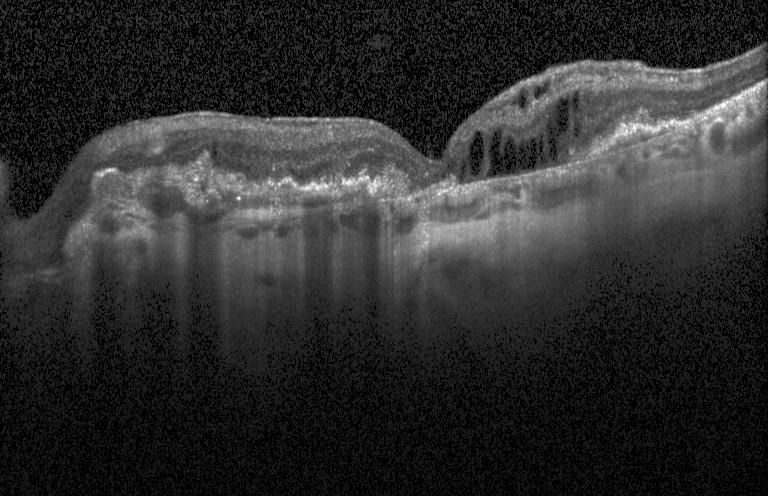

Retinal OCT cross-section. This B-scan demonstrates a choroidal neovascular membrane.